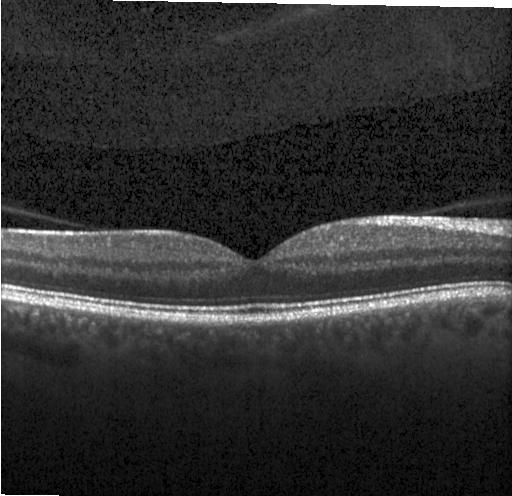

OCT line scan.
Finding: no CNV, no DME, and no drusen.